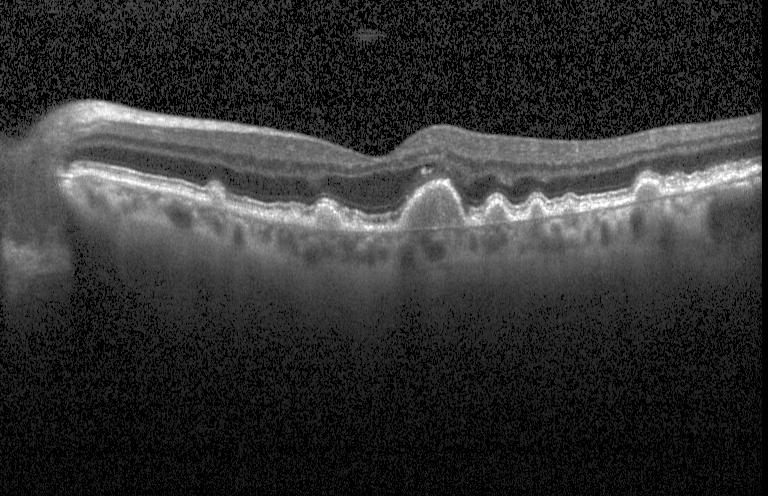 Retinal OCT cross-section showing sub-RPE drusenoid deposits.